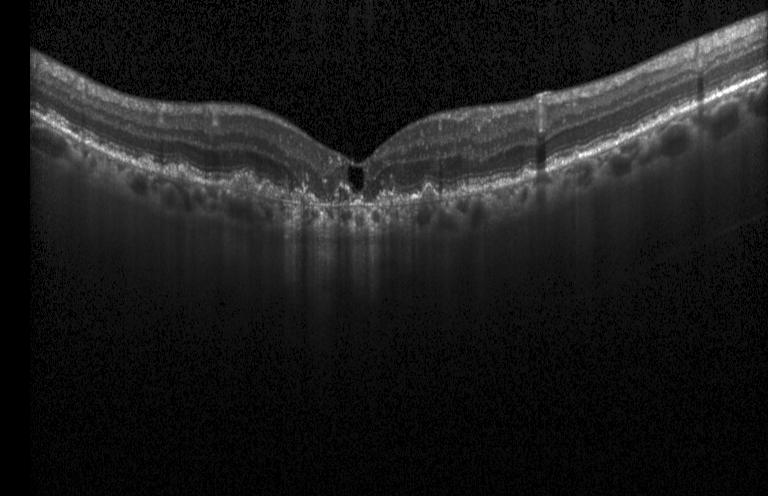

This B-scan demonstrates CNV.